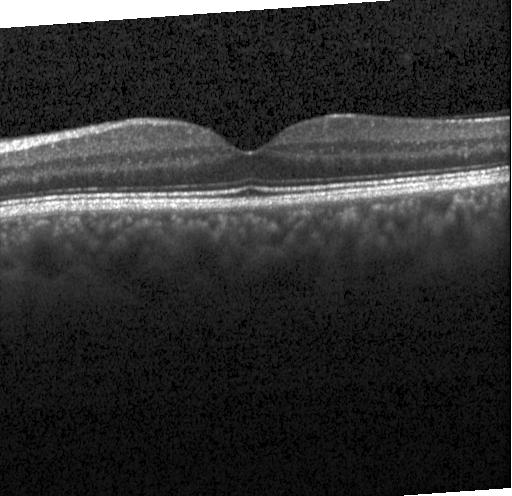

Diagnosis: no evidence of CNV, DME, or drusen.